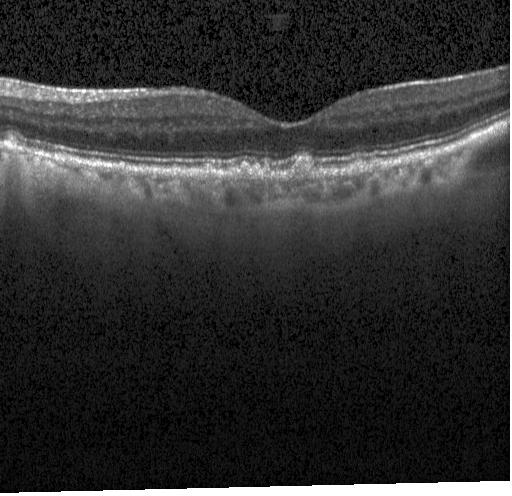 This B-scan demonstrates multiple drusen.